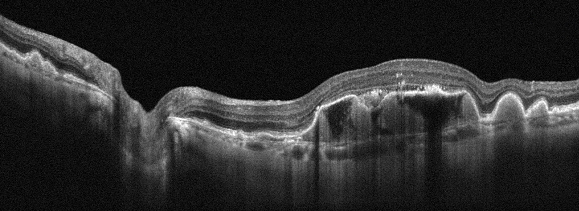 Optical coherence tomography B-scan — Assessment: age-related macular degeneration.